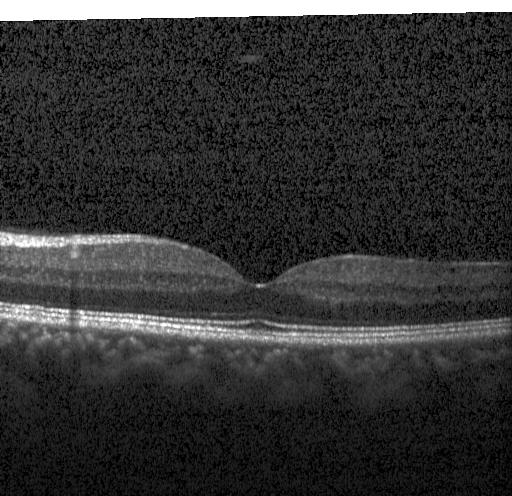
No choroidal neovascularization, no diabetic macular edema, and no drusen.